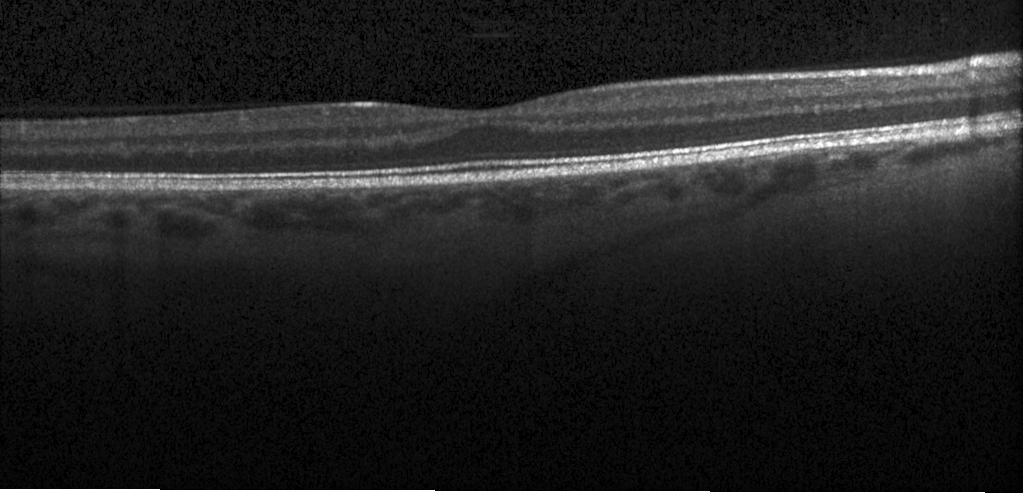

Diagnosis: no evidence of choroidal neovascularization, diabetic macular edema, or drusen.